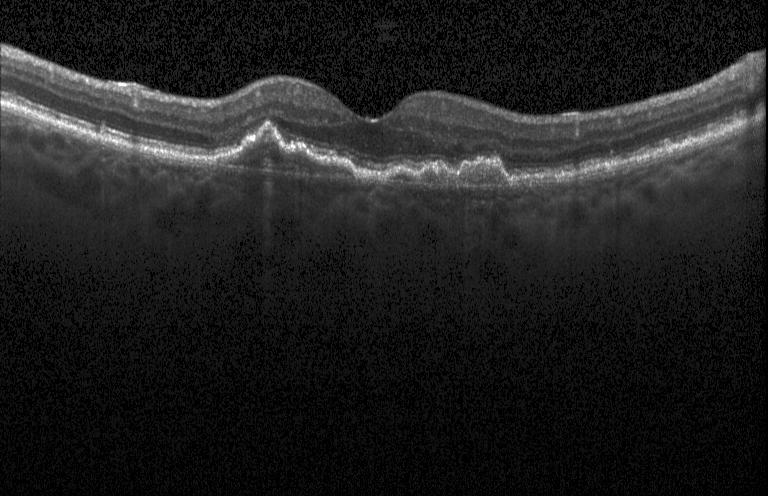
Horizontal scan through the fovea, OCT line scan, acquired on a Heidelberg Spectralis, spectral-domain optical coherence tomography
Finding: a choroidal neovascular membrane.